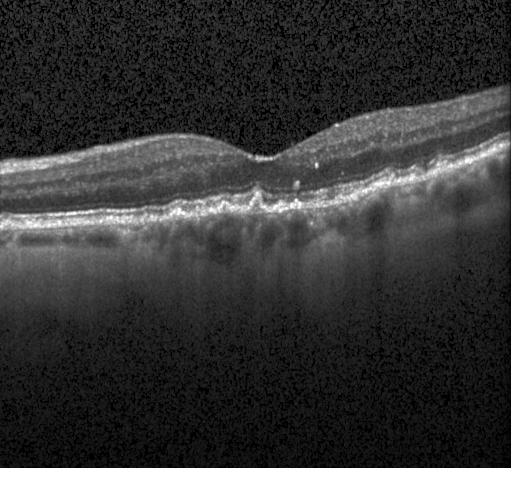 Diagnosis: multiple drusen.